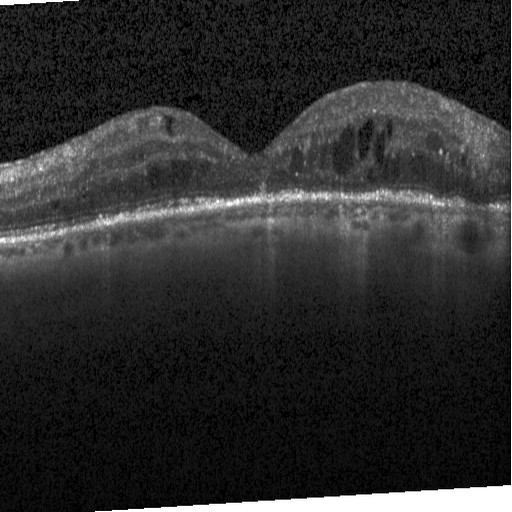

Heidelberg Spectralis; OCT B-scan
Finding: diabetic macular edema (DME).